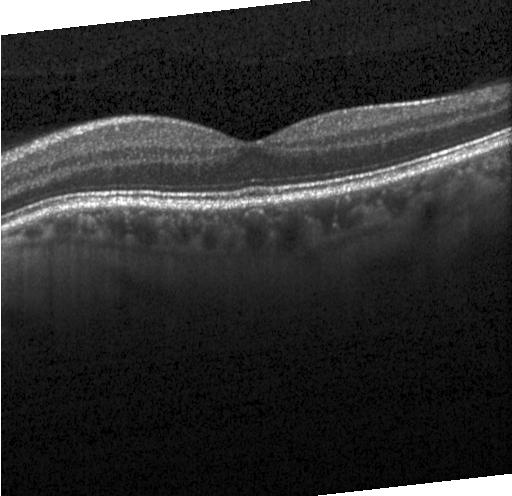

OCT finding: no choroidal neovascularization, diabetic macular edema, or drusen.